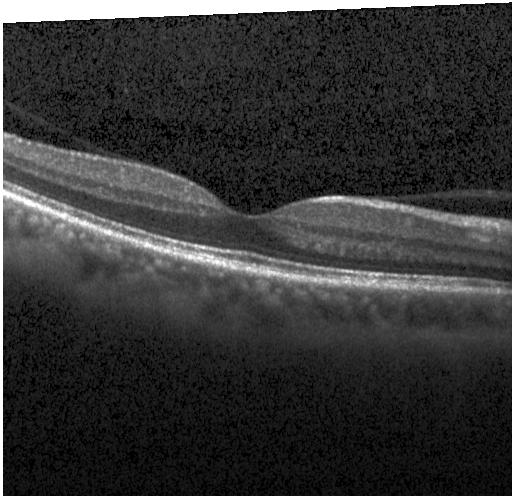 Diagnosis: no choroidal neovascularization, diabetic macular edema, or drusen.